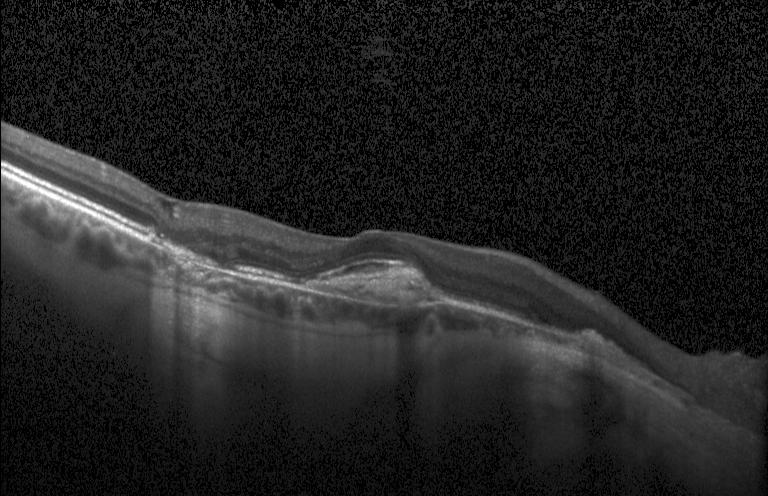
Heidelberg Spectralis; spectral-domain optical coherence tomography; macular scan; OCT line scan.
Diagnosis: a choroidal neovascular membrane.